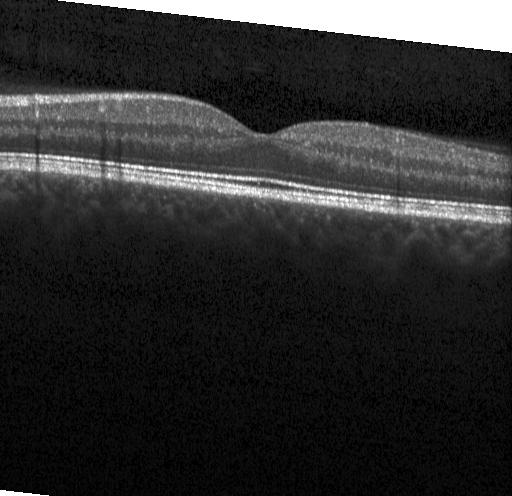
No choroidal neovascularization, no diabetic macular edema, and no drusen.